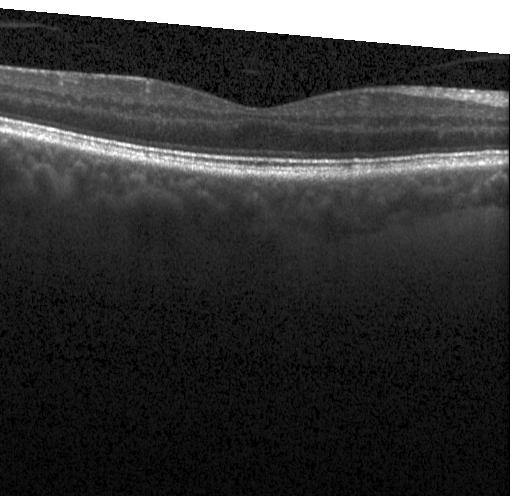 OCT B-scan — OCT finding: neither choroidal neovascularization, diabetic macular edema, nor drusen.